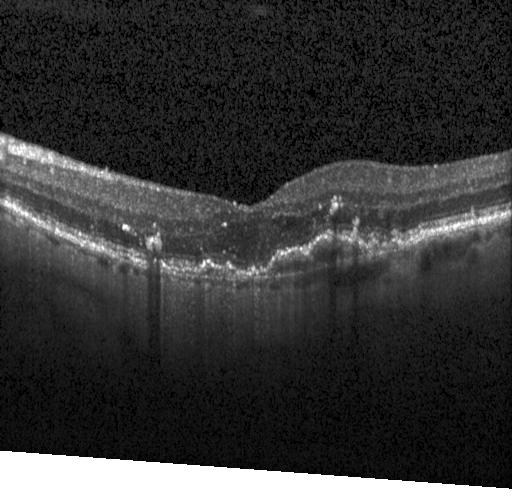
Heidelberg Spectralis; retinal OCT B-scan; through the macula.
This B-scan demonstrates choroidal neovascularization.